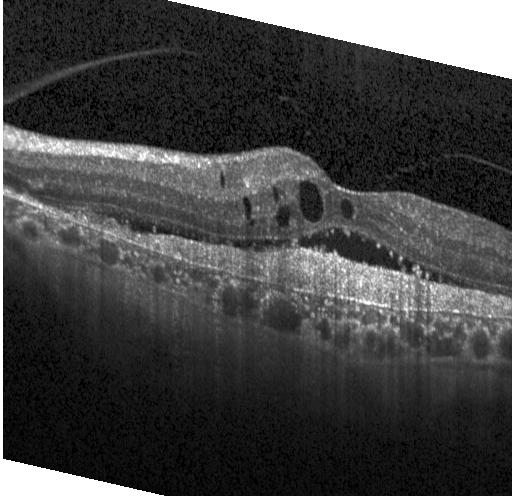

Dx: choroidal neovascularization.